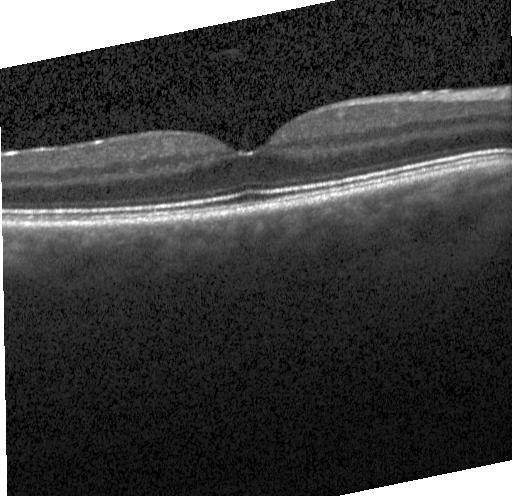
Heidelberg Spectralis; macular scan; SD-OCT; retinal OCT B-scan.
No evidence of CNV, DME, or drusen.